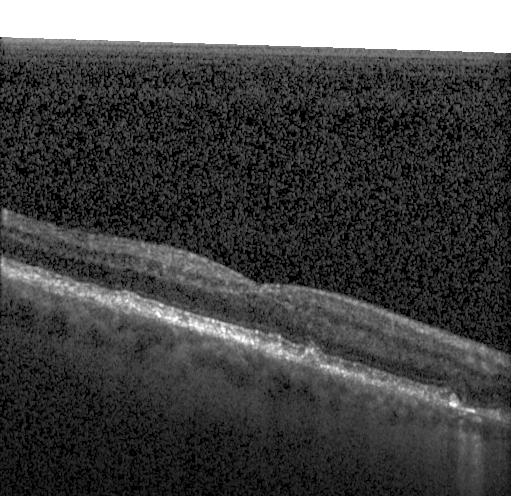
Heidelberg Spectralis; OCT B-scan; SD-OCT
This B-scan demonstrates sub-RPE drusenoid deposits.